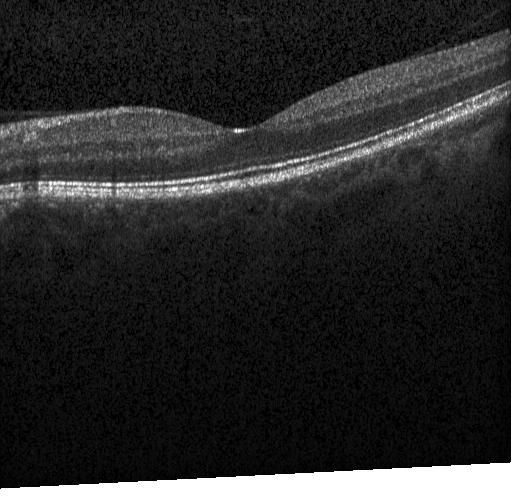
Retinal OCT cross-section. Macular OCT: no CNV, no DME, and no drusen.